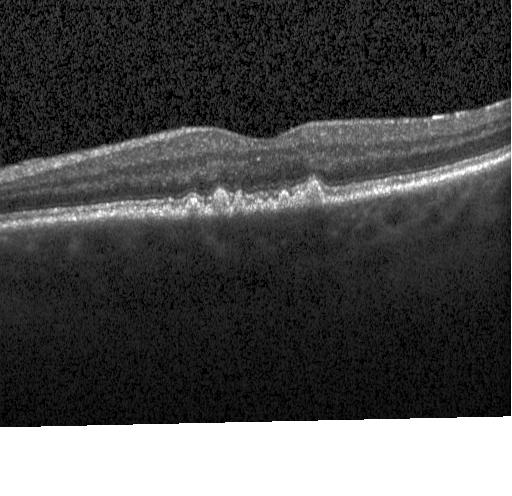

Macular scan. OCT line scan. Heidelberg Spectralis
Impression: sub-RPE drusenoid deposits.